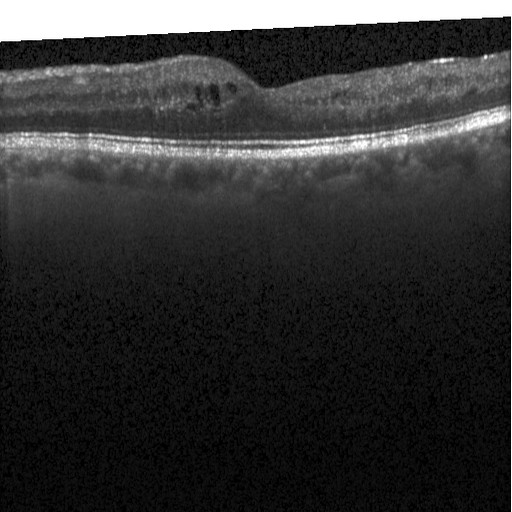

Finding: DME.